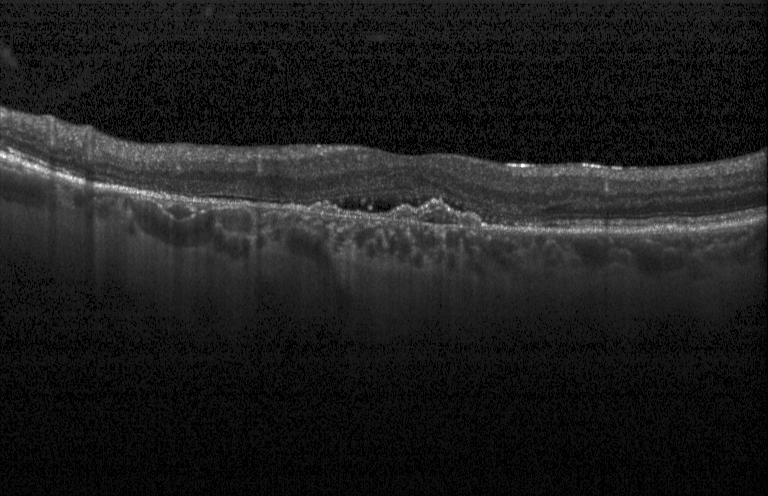 Macular OCT: choroidal neovascularization.